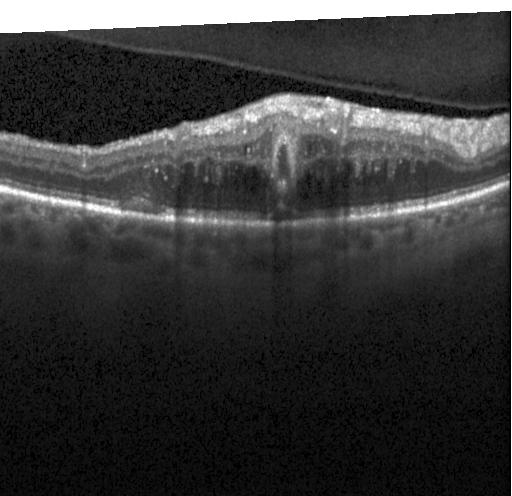

SD-OCT; optical coherence tomography scan.
Choroidal neovascularization.